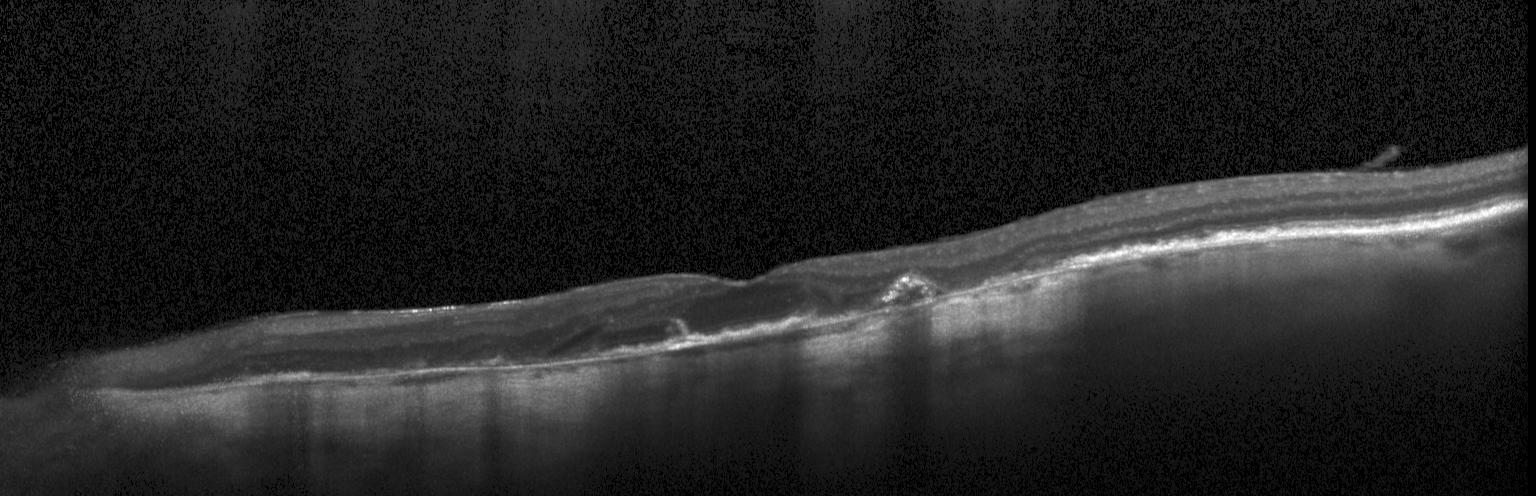 OCT scan showing choroidal neovascularization.